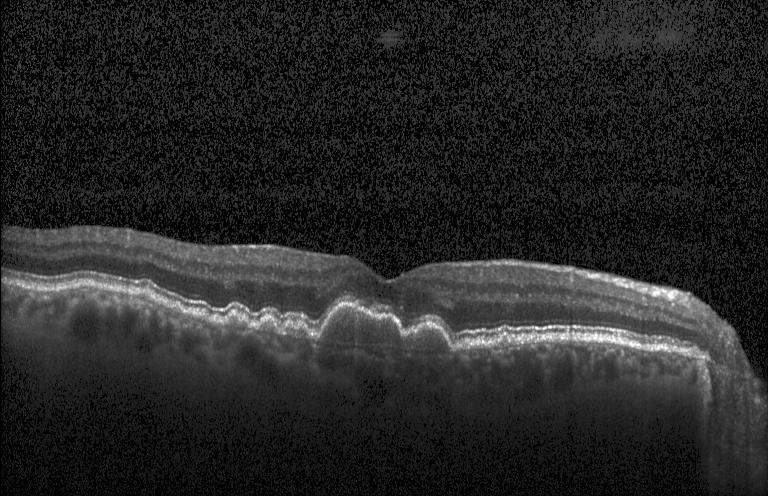

Fovea-centered, optical coherence tomography scan, Heidelberg Spectralis OCT system.
This B-scan demonstrates sub-RPE drusenoid deposits.